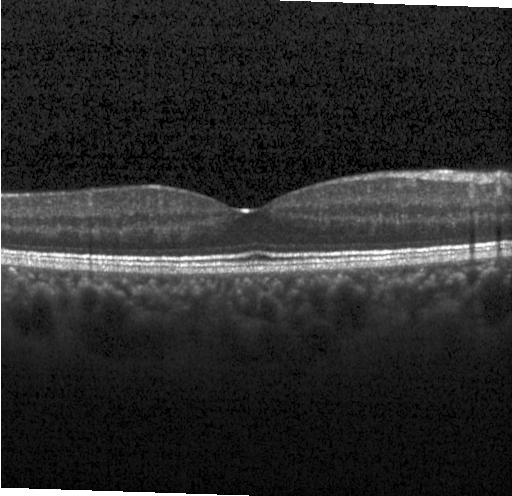
Heidelberg Spectralis OCT system · macular scan · SD-OCT · OCT B-scan
This B-scan demonstrates no choroidal neovascularization, diabetic macular edema, or drusen.